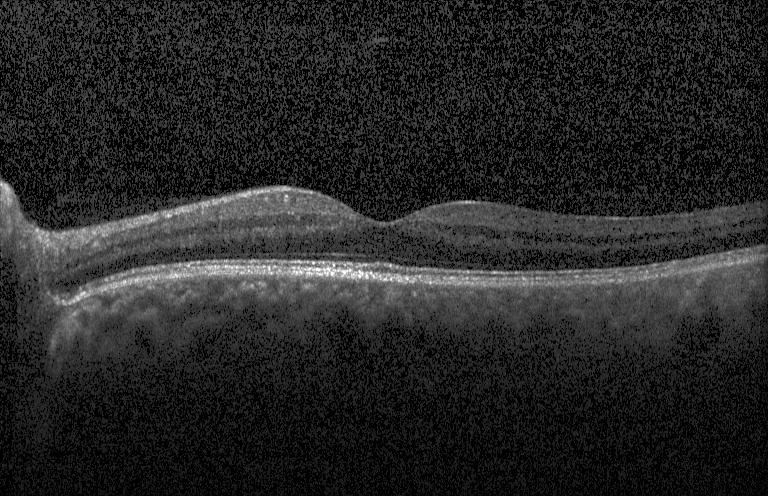

OCT line scan.
Diagnosis: neither choroidal neovascularization, diabetic macular edema, nor drusen.